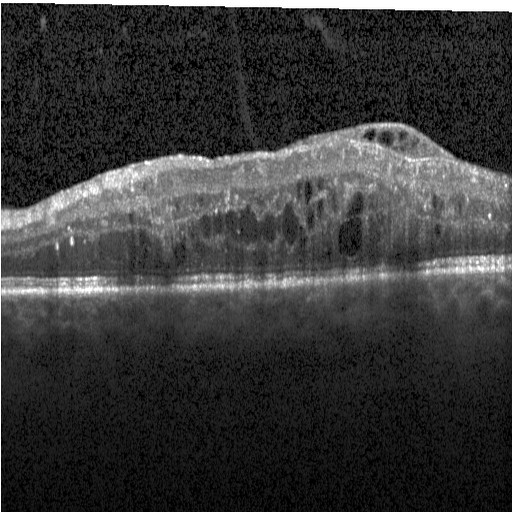
Spectral-domain OCT B-scan: diabetic macular edema (DME).